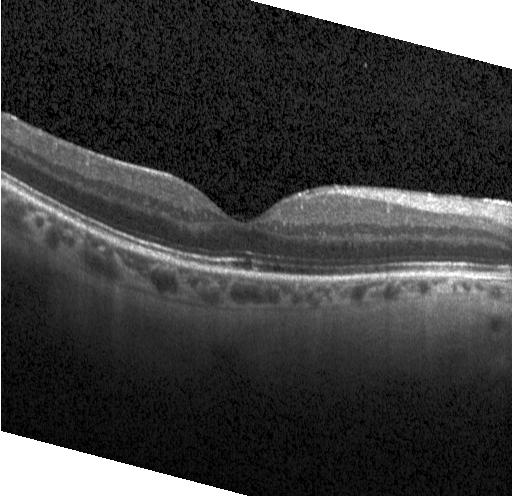

OCT line scan · centered on the fovea · acquired on a Heidelberg Spectralis — Diagnosis: no CNV, DME, or drusen.